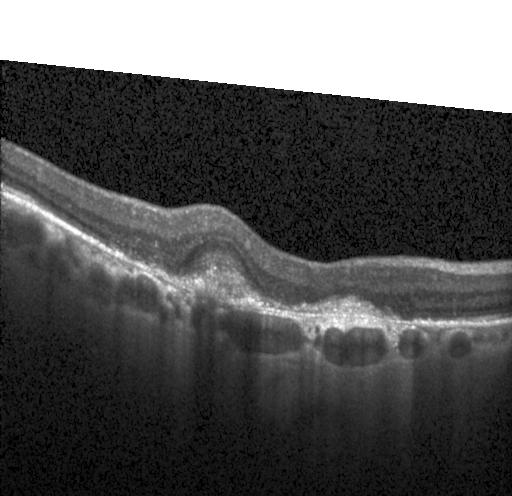

OCT line scan · Heidelberg Spectralis · SD-OCT. The scan shows choroidal neovascularization (CNV).